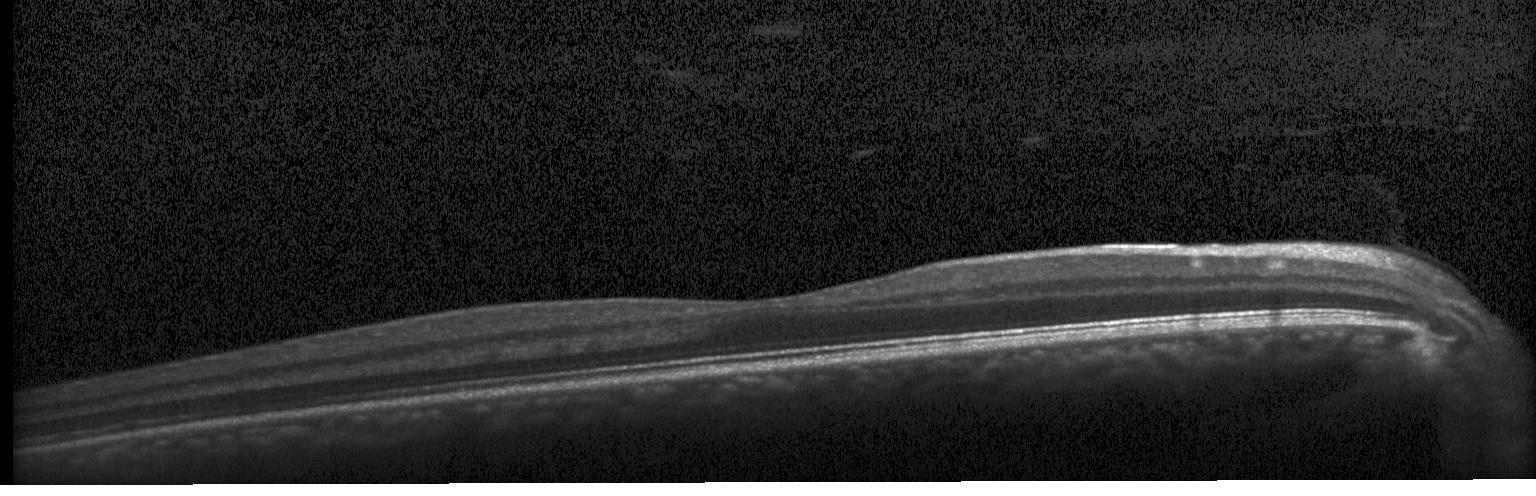
OCT B-scan. The scan shows no choroidal neovascularization, diabetic macular edema, or drusen.